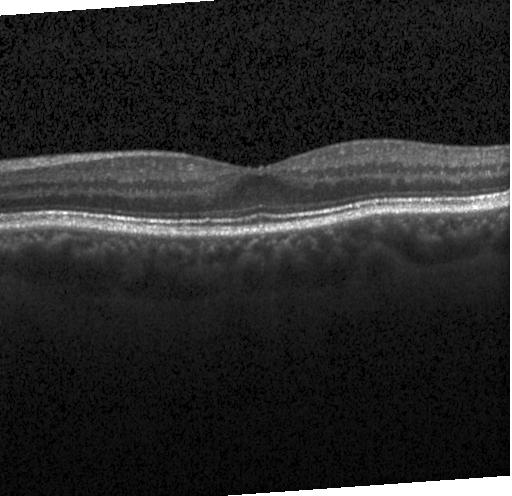

This B-scan demonstrates no evidence of choroidal neovascularization, diabetic macular edema, or drusen.